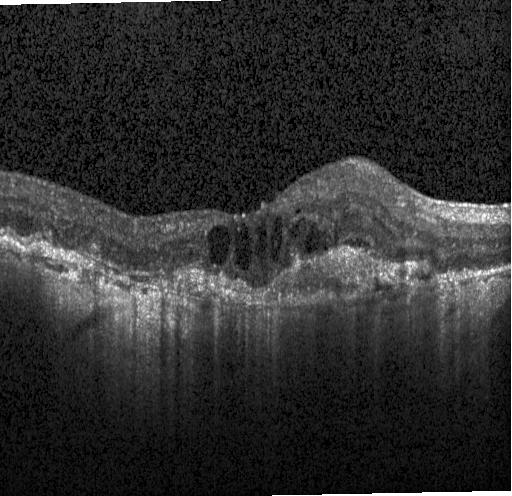

Impression: choroidal neovascularization (CNV).